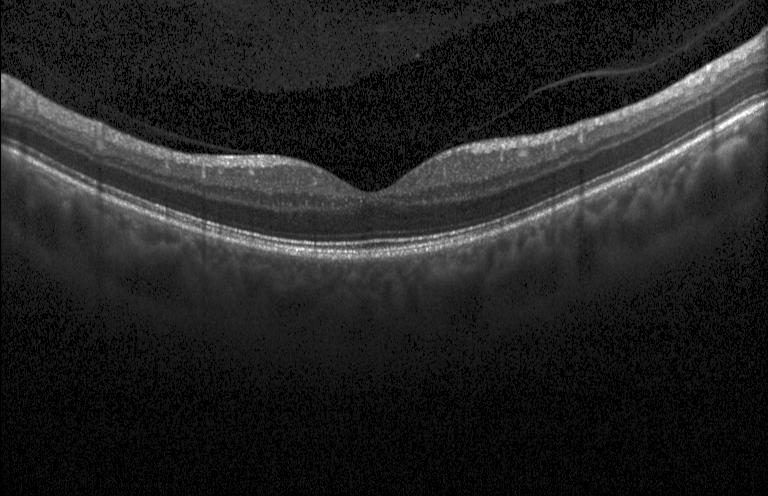
Retinal OCT B-scan.
Macular OCT: no CNV, no DME, and no drusen.